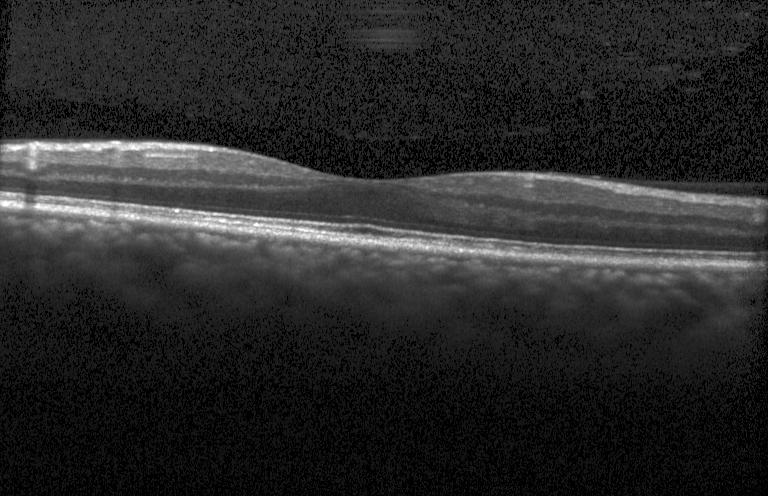
OCT line scan, fovea-centered, Heidelberg Spectralis, spectral-domain optical coherence tomography — Assessment: no choroidal neovascularization, no diabetic macular edema, and no drusen.